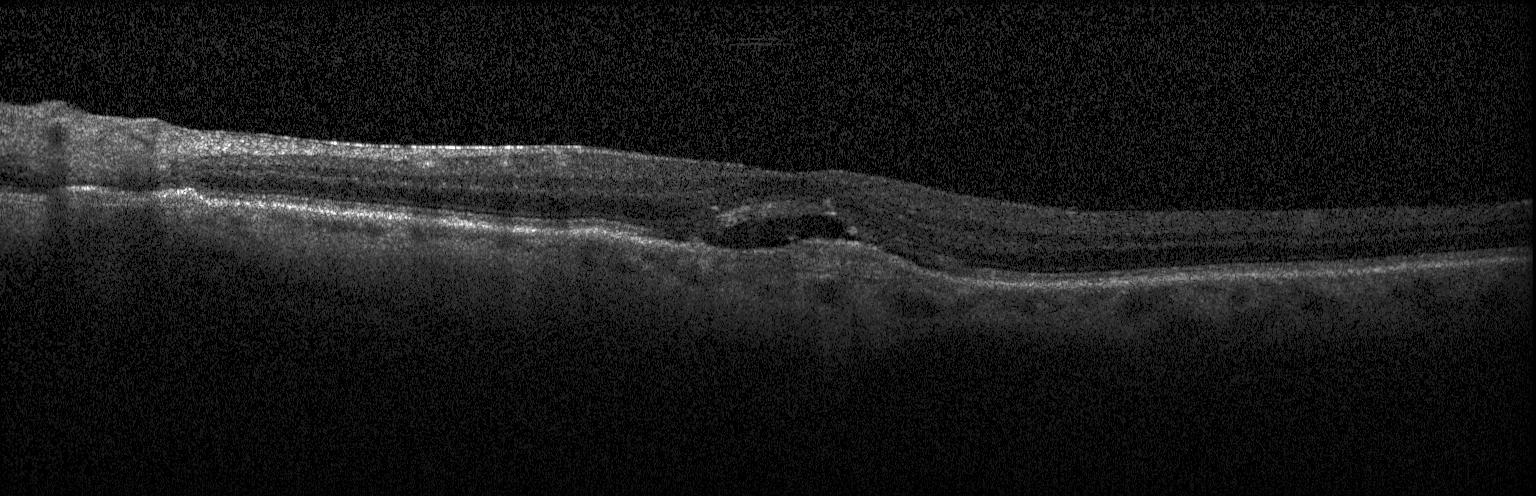 OCT scan showing a choroidal neovascular membrane.